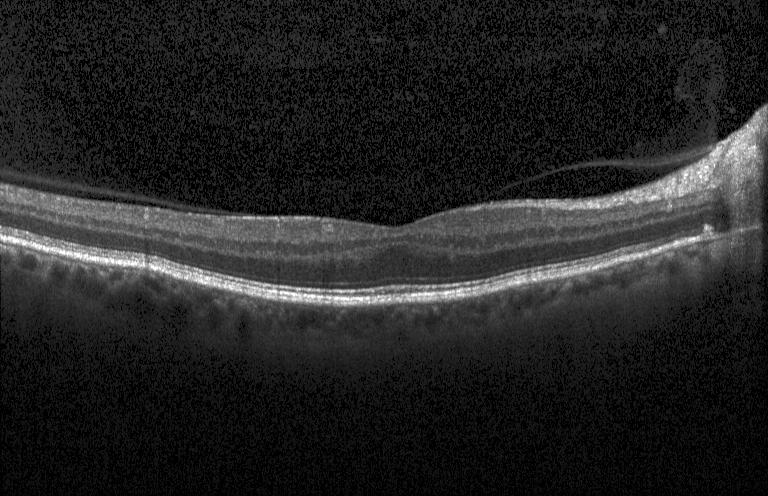

Optical coherence tomography B-scan, Heidelberg Spectralis
The scan shows no CNV, DME, or drusen.